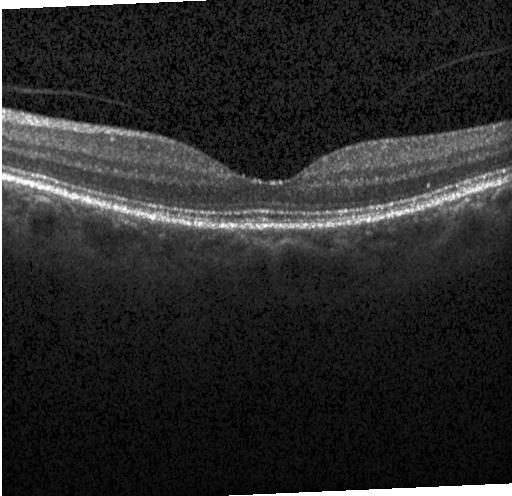 Diagnosis: neither CNV, DME, nor drusen.